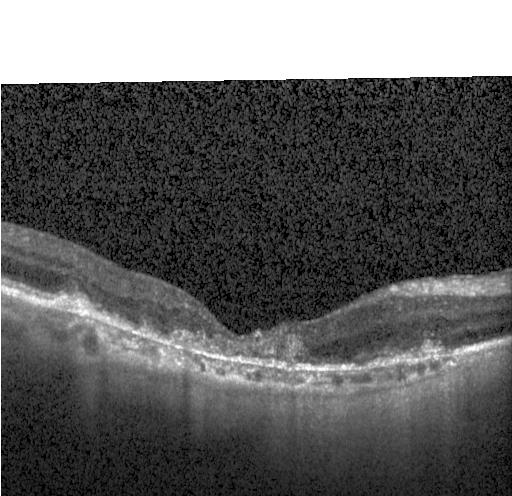
The scan shows choroidal neovascularization.